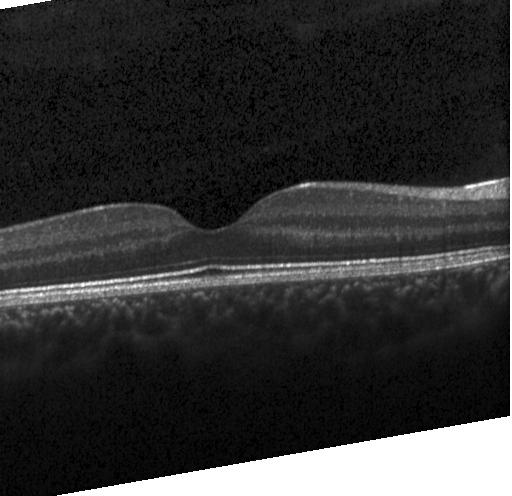 OCT line scan. Heidelberg Spectralis OCT system.
Assessment: no choroidal neovascularization, diabetic macular edema, or drusen.